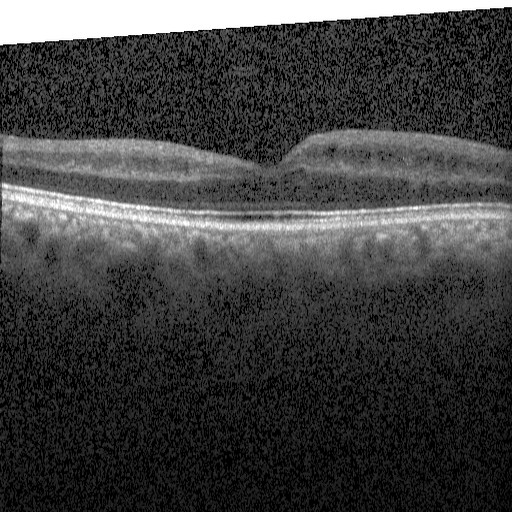
Optical coherence tomography scan, SD-OCT, fovea-centered. The scan shows DME.